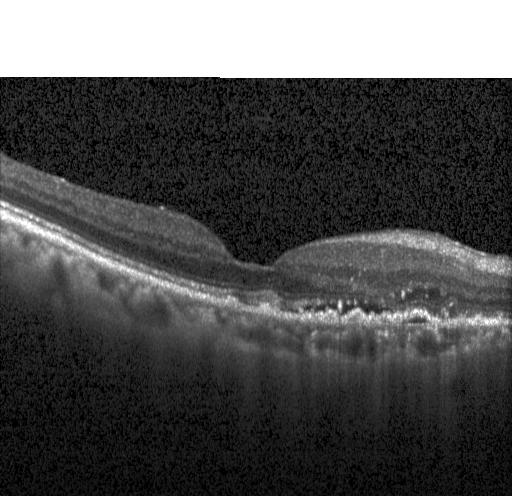
Through the macula. Spectral-domain OCT. Optical coherence tomography scan
Choroidal neovascularization (CNV).